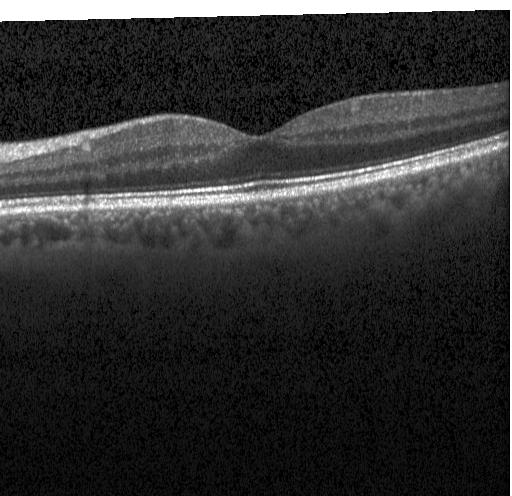
Acquired on a Heidelberg Spectralis. Spectral-domain optical coherence tomography. Horizontal scan through the fovea. OCT B-scan — Dx: no choroidal neovascularization, no diabetic macular edema, and no drusen.